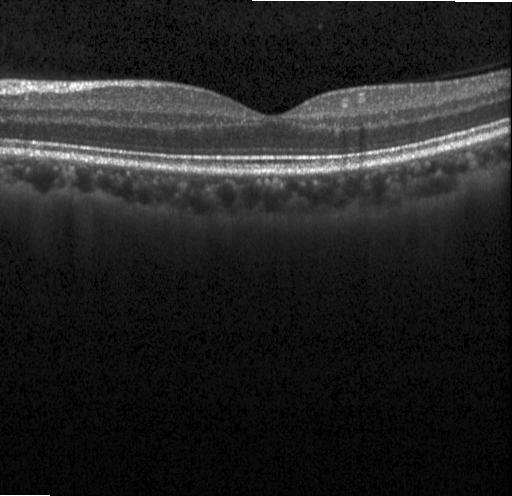
OCT B-scan. Acquired on a Heidelberg Spectralis. SD-OCT — Finding: no choroidal neovascularization, diabetic macular edema, or drusen.